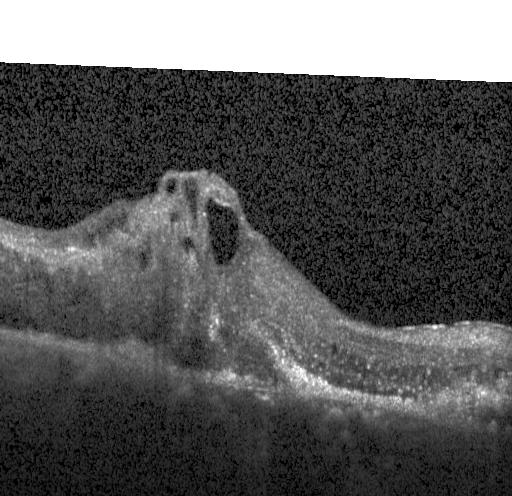

Optical coherence tomography B-scan · macular scan
Diagnosis: CNV.